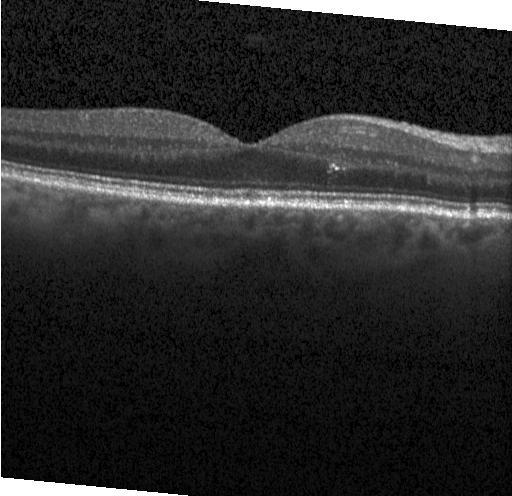

Spectral-domain optical coherence tomography · OCT line scan · Heidelberg Spectralis OCT system. Finding: neither choroidal neovascularization, diabetic macular edema, nor drusen.